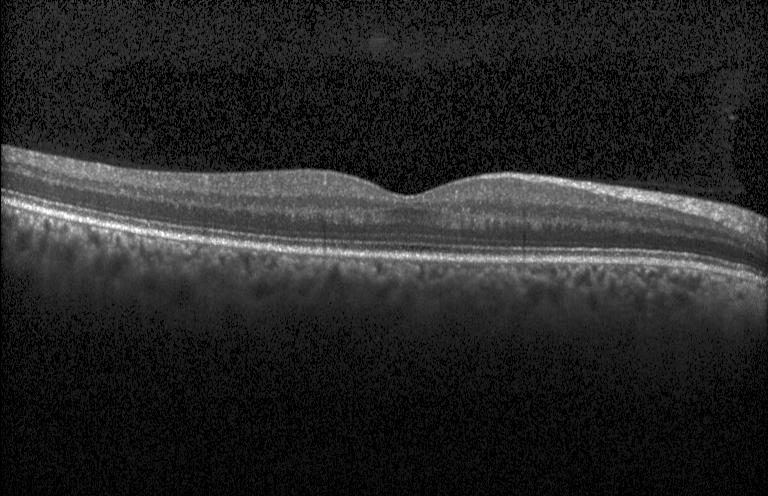

Spectral-domain optical coherence tomography · centered on the fovea · OCT B-scan.
Assessment: no evidence of choroidal neovascularization, diabetic macular edema, or drusen.